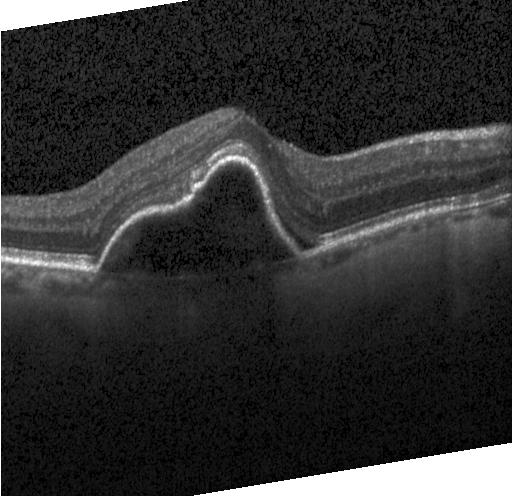 Retinal OCT cross-section. Fovea-centered. Finding: a choroidal neovascular membrane.